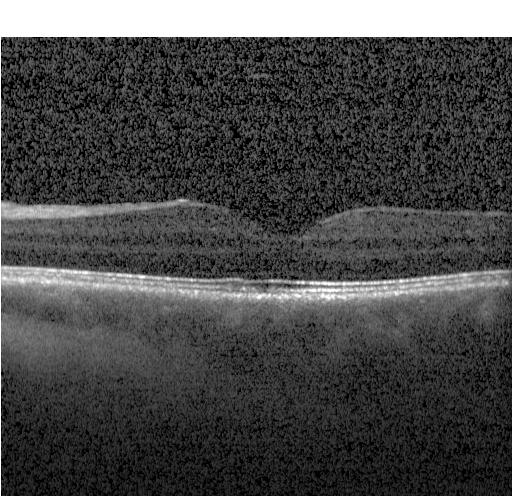
Finding: neither CNV, DME, nor drusen.